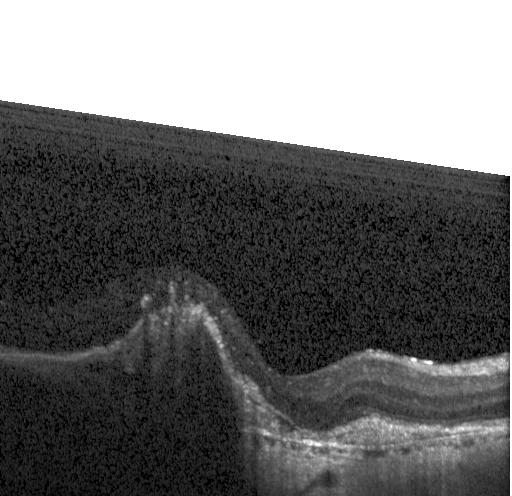
OCT B-scan · spectral-domain optical coherence tomography · through the macula — This B-scan demonstrates a choroidal neovascular membrane.